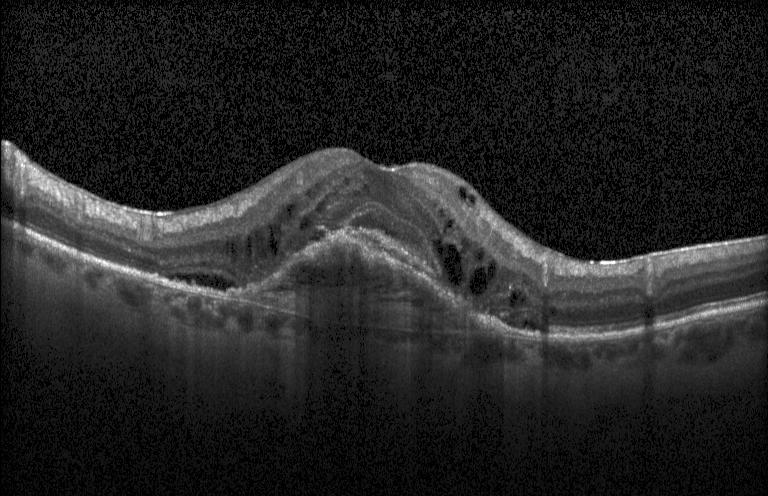

OCT B-scan
Dx: choroidal neovascularization (CNV).